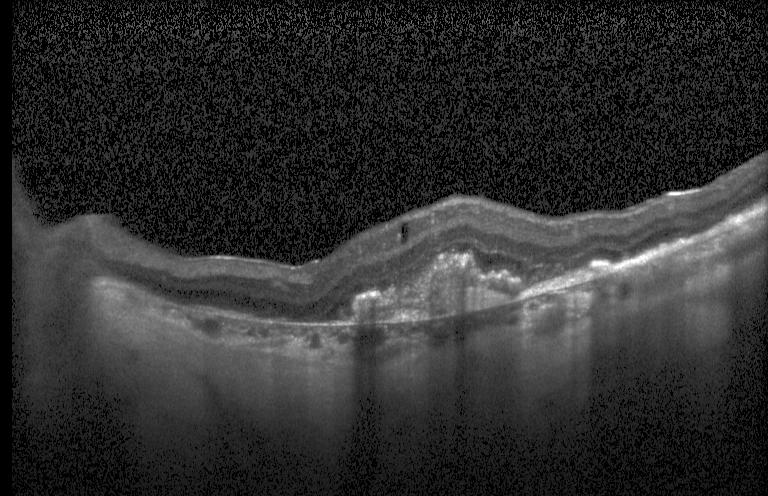

Heidelberg Spectralis OCT system, through the macula, optical coherence tomography B-scan.
Finding: a choroidal neovascular membrane.